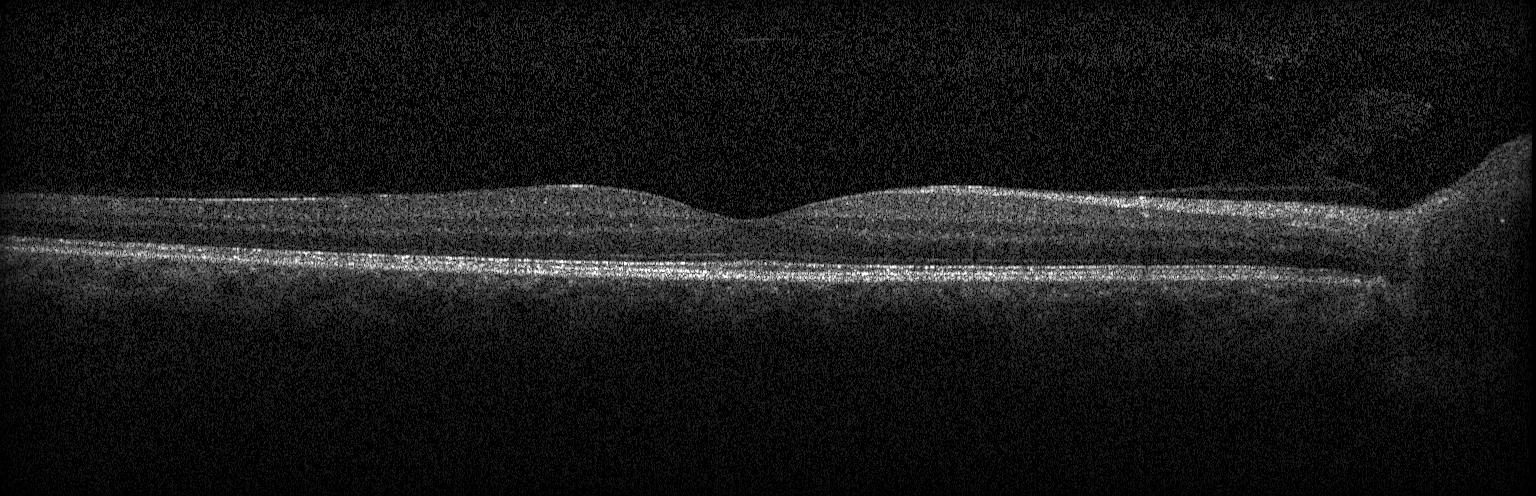
Finding: neither CNV, DME, nor drusen.